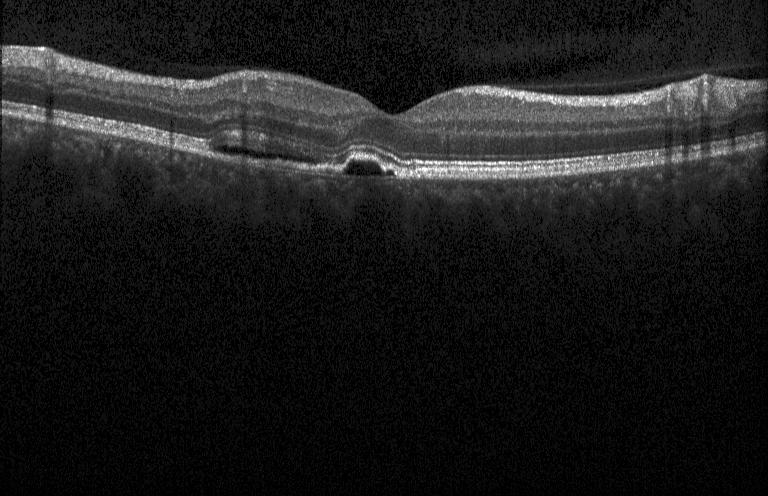
Macular OCT: a choroidal neovascular membrane.